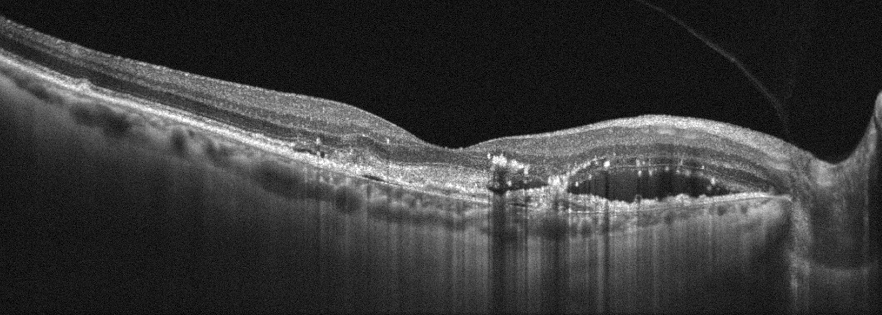

Optical coherence tomography B-scan; OD — The scan shows age-related macular degeneration (AMD).